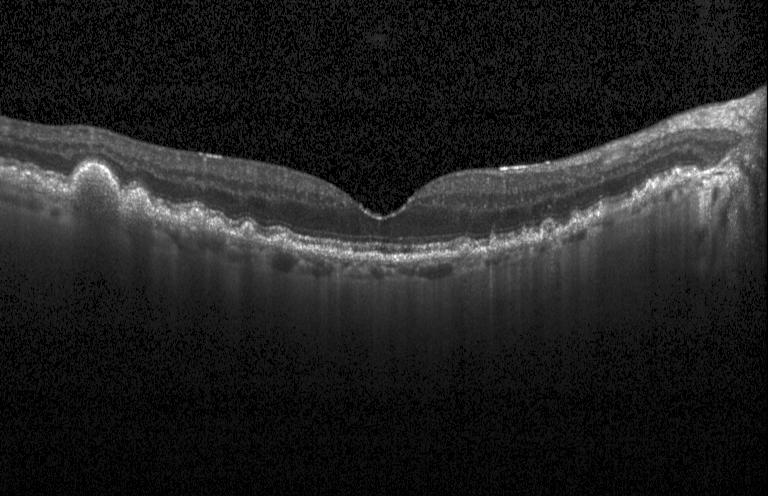 OCT B-scan showing drusen.